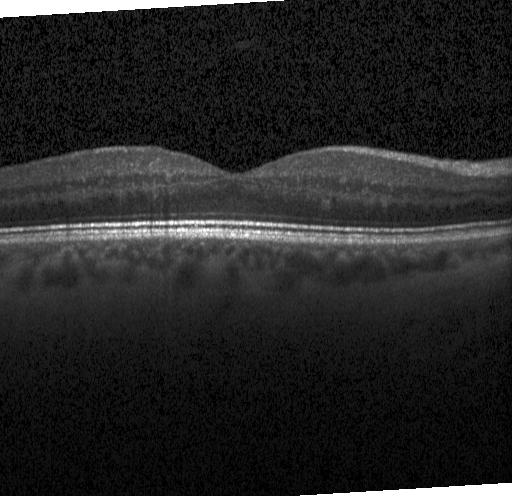

Retinal OCT cross-section showing no evidence of CNV, DME, or drusen.